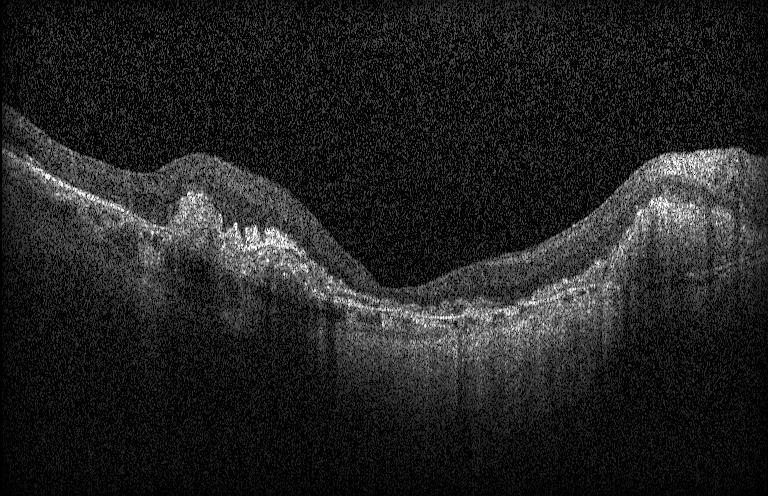
OCT B-scan showing a choroidal neovascular membrane.